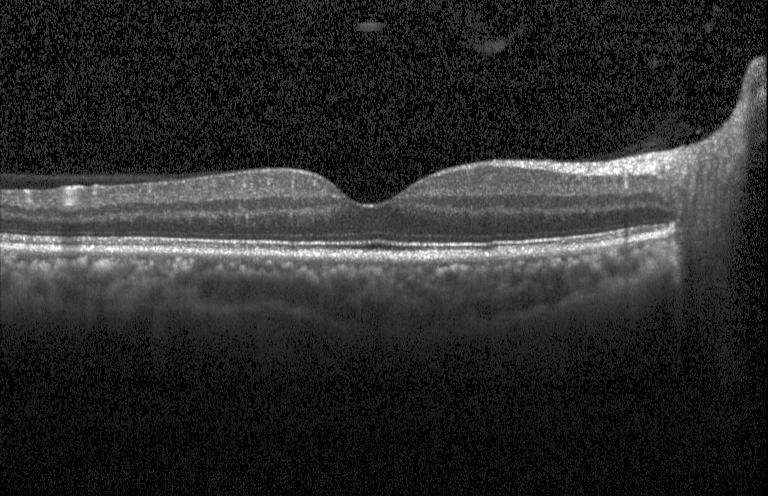 Finding: no CNV, DME, or drusen.